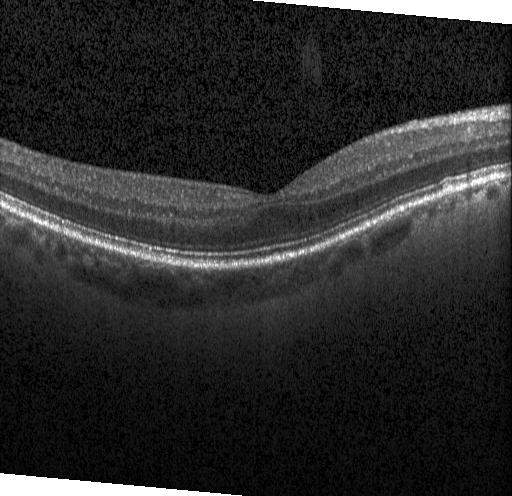 OCT B-scan, Heidelberg Spectralis, horizontal scan through the fovea.
Impression: neither choroidal neovascularization, diabetic macular edema, nor drusen.